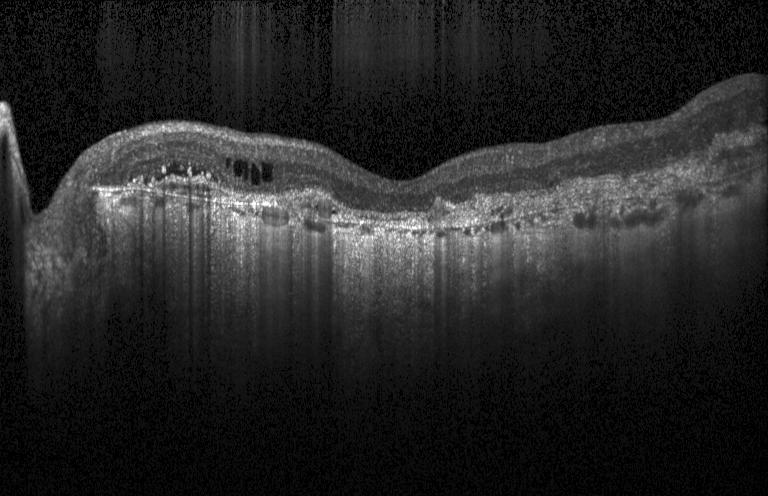
Retinal OCT cross-section · Heidelberg Spectralis OCT system · spectral-domain optical coherence tomography. Choroidal neovascularization (CNV).